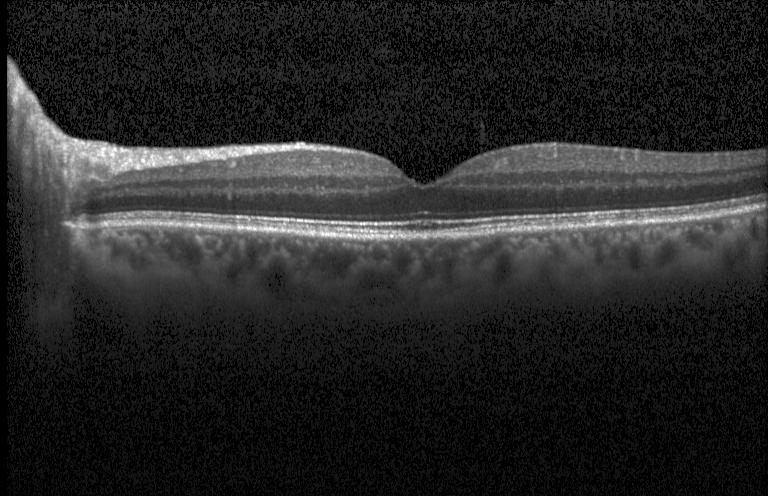
Retinal OCT B-scan, fovea-centered.
OCT finding: no CNV, no DME, and no drusen.